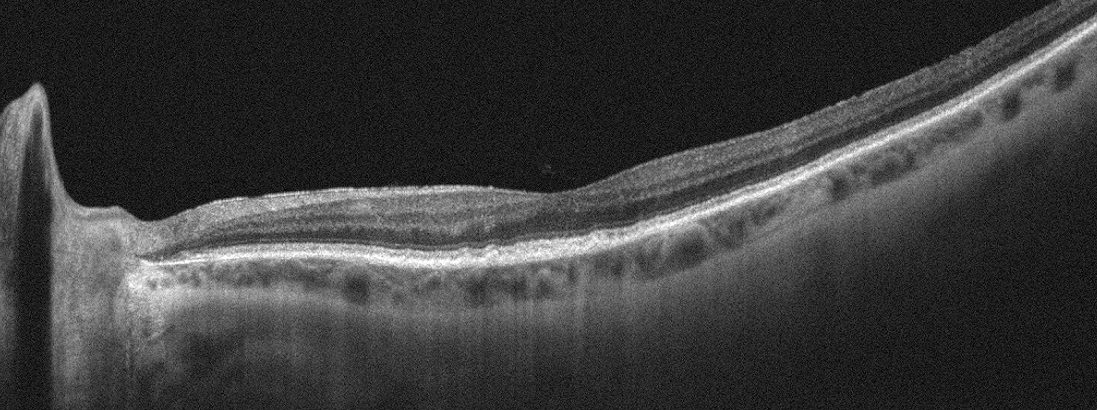

Optical coherence tomography scan — This B-scan demonstrates AMD.